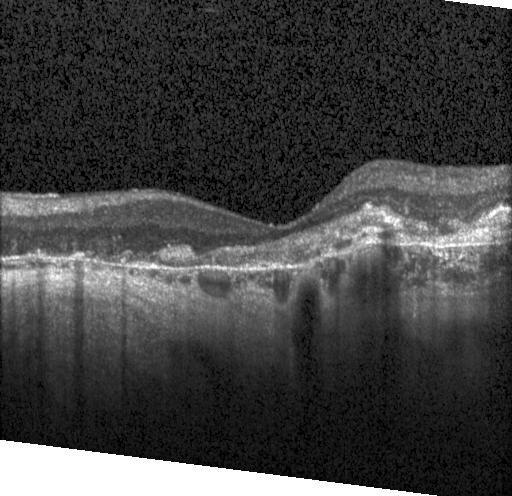 Spectral-domain OCT; acquired on a Heidelberg Spectralis; fovea-centered; optical coherence tomography B-scan. Impression: a choroidal neovascular membrane.